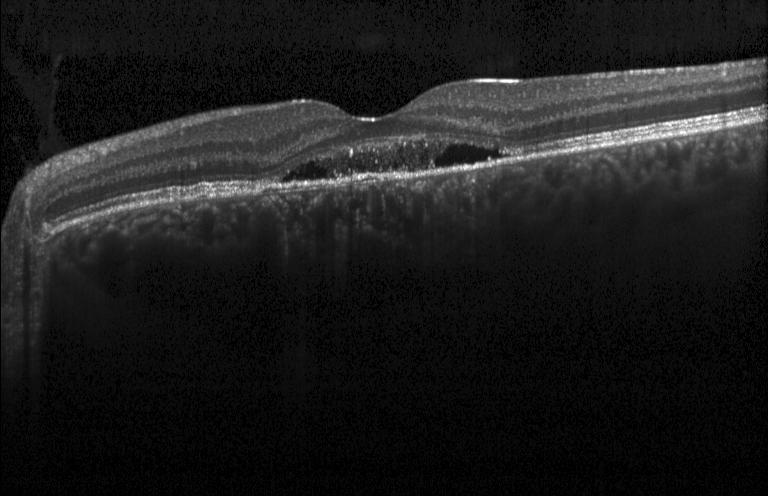

Optical coherence tomography scan, spectral-domain OCT.
OCT finding: a choroidal neovascular membrane.